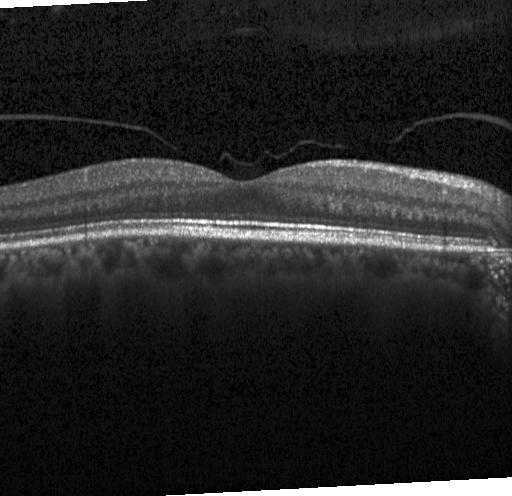 OCT line scan; spectral-domain OCT; centered on the fovea
Finding: no evidence of choroidal neovascularization, diabetic macular edema, or drusen.